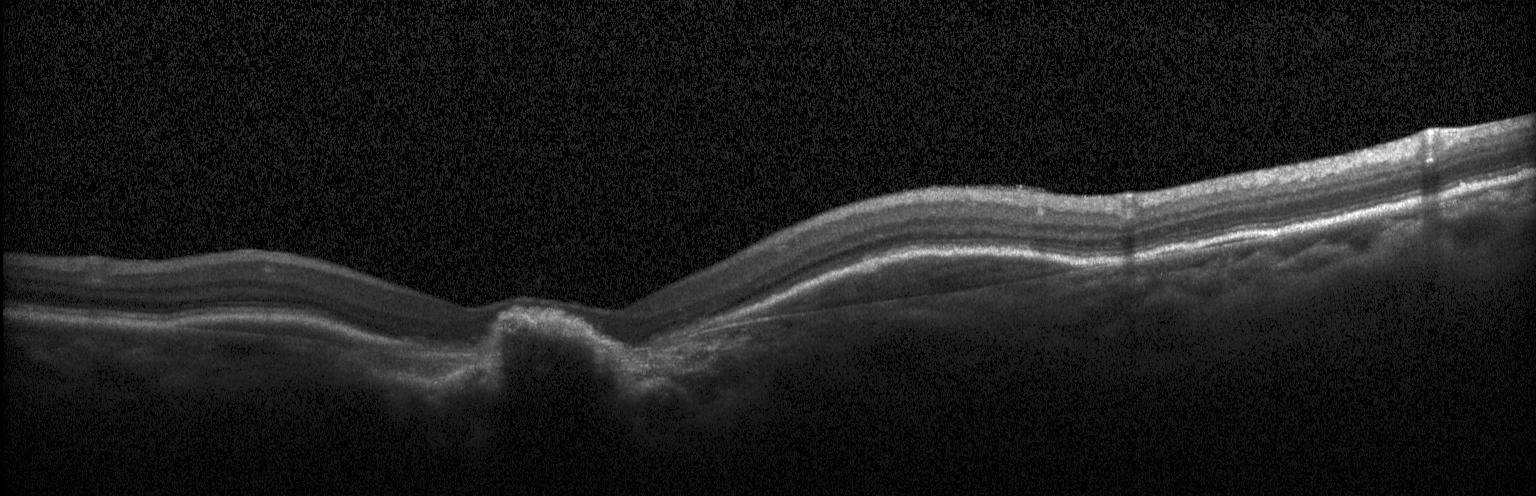
A choroidal neovascular membrane.